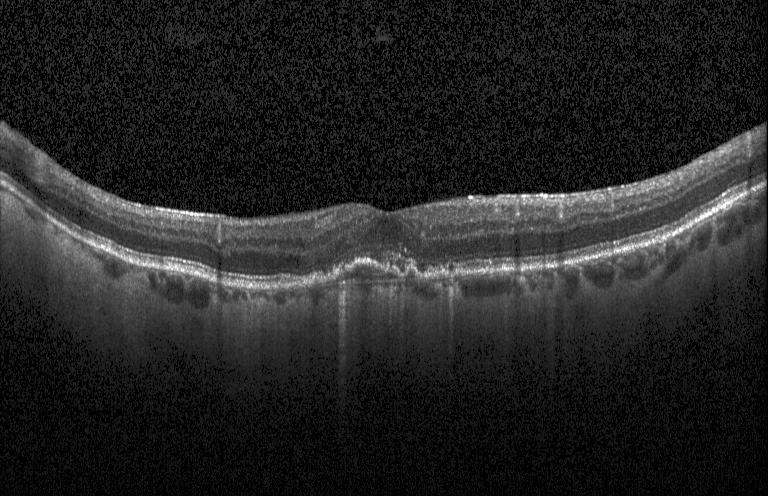
Retinal OCT cross-section
Diagnosis: a choroidal neovascular membrane.